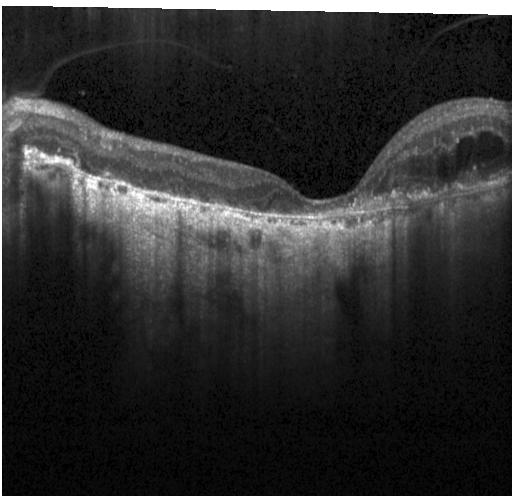
Optical coherence tomography scan.
The scan shows choroidal neovascularization (CNV).